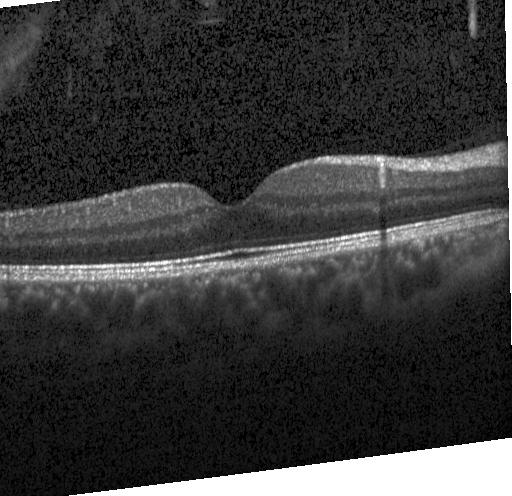

Optical coherence tomography B-scan; macular scan; acquired on a Heidelberg Spectralis; spectral-domain OCT
Dx: no CNV, DME, or drusen.